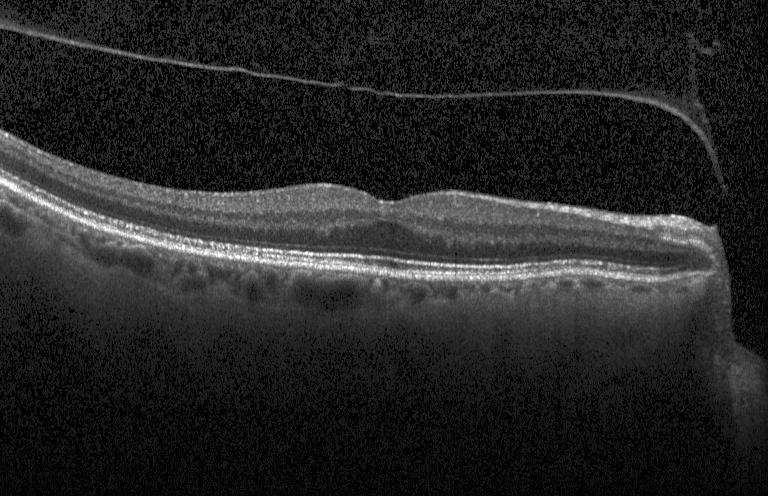

Acquired on a Heidelberg Spectralis, macular scan, OCT line scan, SD-OCT. Finding: no choroidal neovascularization, no diabetic macular edema, and no drusen.